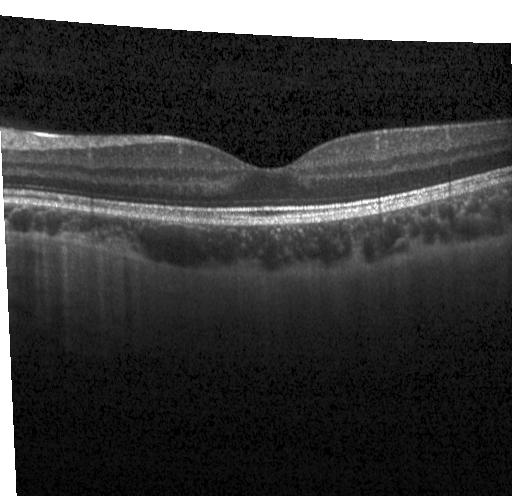 Heidelberg Spectralis. Spectral-domain optical coherence tomography. Retinal OCT cross-section. Centered on the fovea. Diagnosis: no evidence of choroidal neovascularization, diabetic macular edema, or drusen.